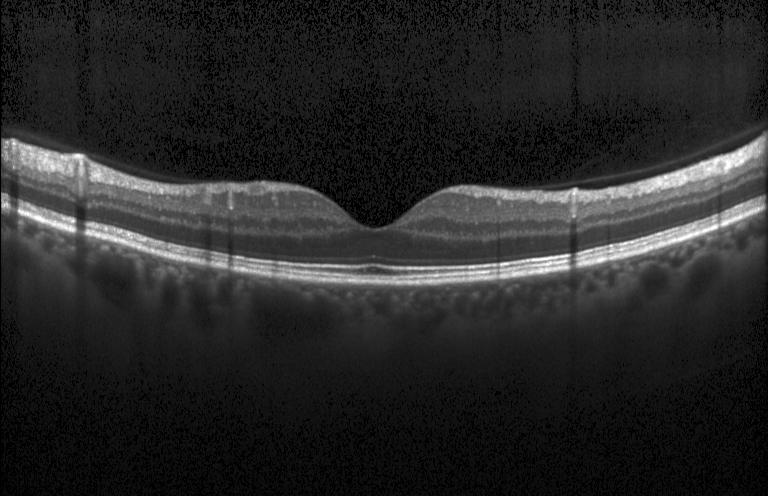

OCT line scan.
Impression: neither CNV, DME, nor drusen.